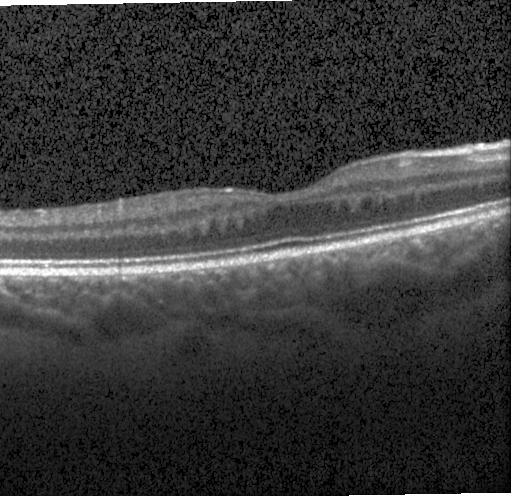

Heidelberg Spectralis. OCT line scan
No CNV, DME, or drusen.